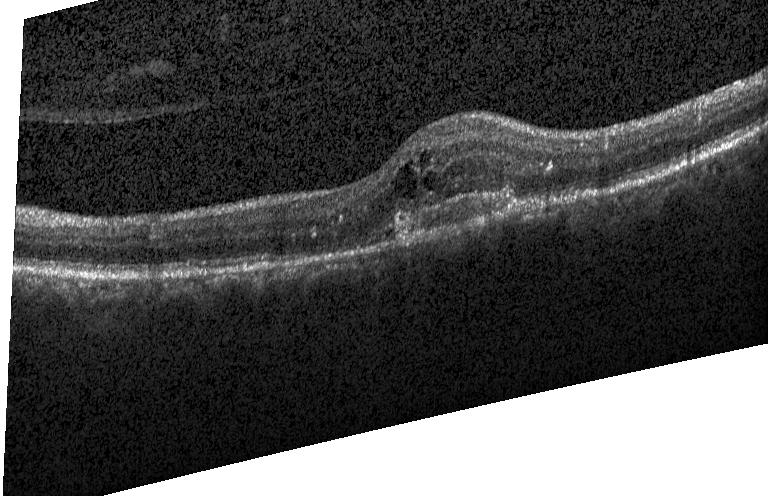
Macular OCT: a choroidal neovascular membrane.